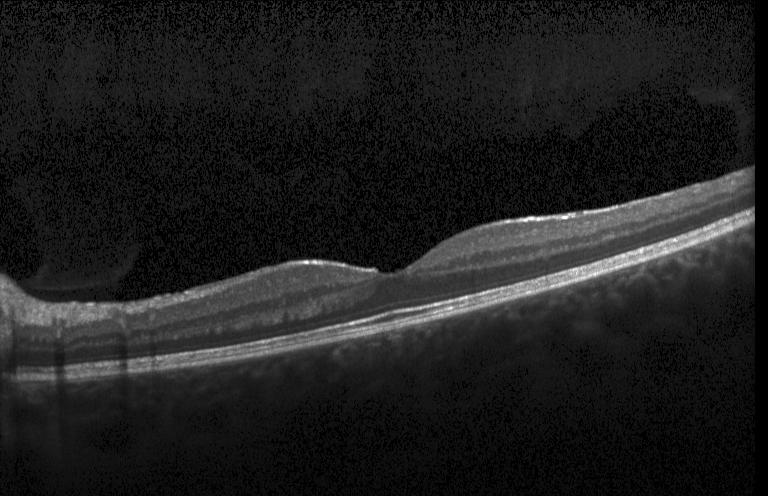 Retinal OCT cross-section showing neither choroidal neovascularization, diabetic macular edema, nor drusen.